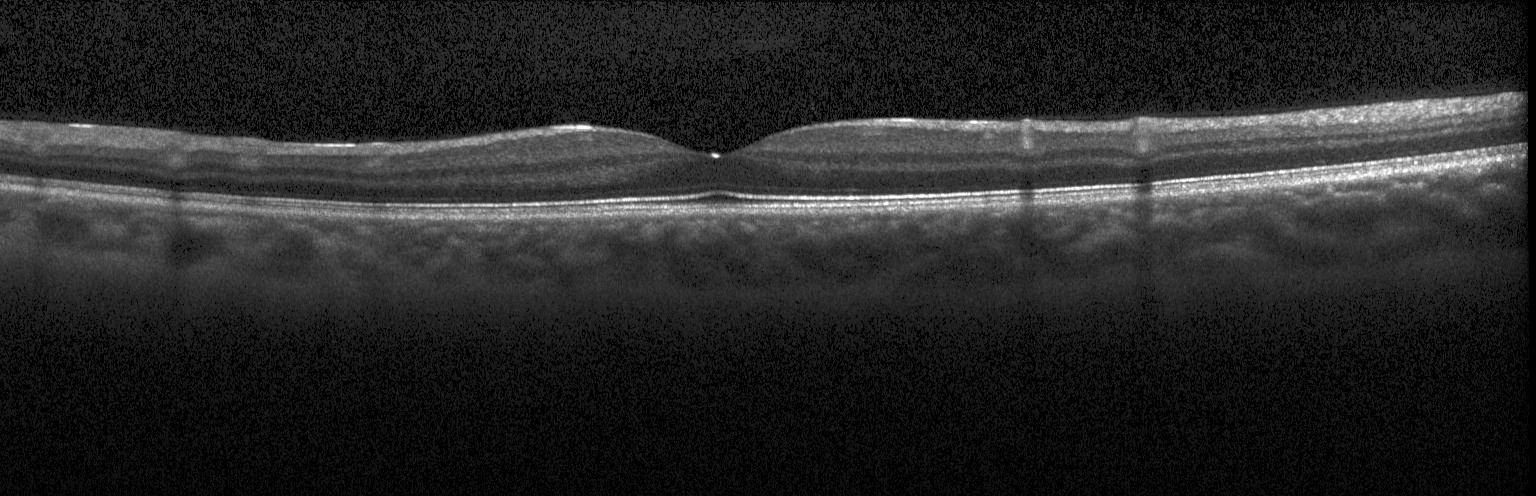
Spectral-domain OCT B-scan: no choroidal neovascularization, no diabetic macular edema, and no drusen.